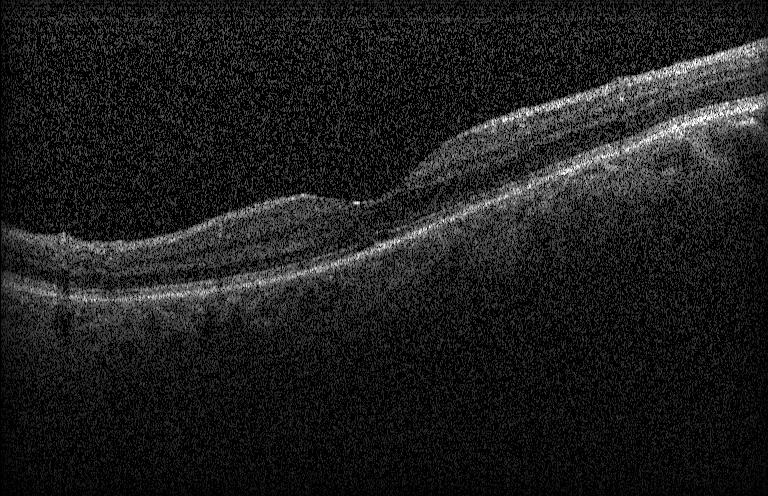
SD-OCT. Horizontal scan through the fovea. Heidelberg Spectralis. Retinal OCT B-scan
OCT finding: no choroidal neovascularization, no diabetic macular edema, and no drusen.